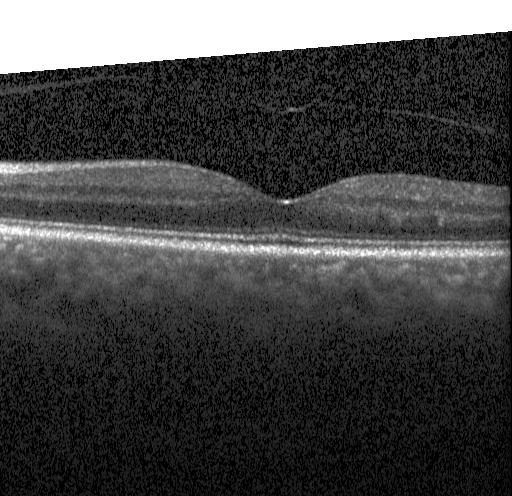 OCT line scan.
The scan shows no evidence of CNV, DME, or drusen.